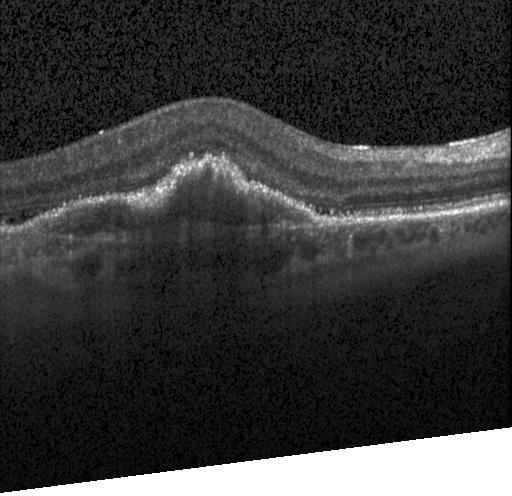
Horizontal scan through the fovea · retinal OCT cross-section. Diagnosis: a choroidal neovascular membrane.